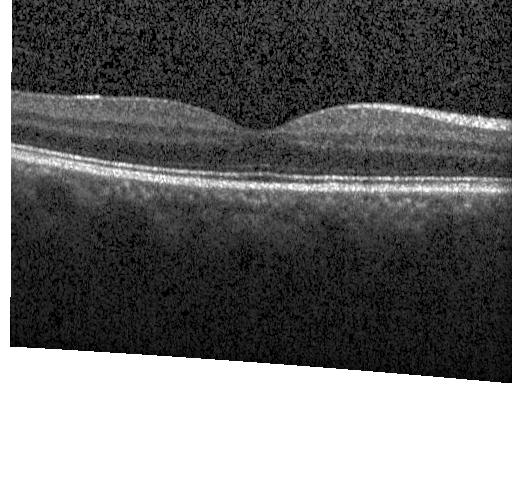
Instrument: Heidelberg Spectralis · optical coherence tomography scan.
Diagnosis: no CNV, no DME, and no drusen.